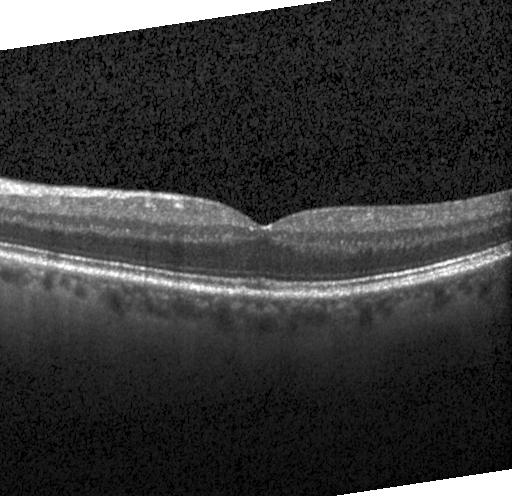 Instrument: Heidelberg Spectralis · through the macula · spectral-domain optical coherence tomography · retinal OCT cross-section — Impression: neither CNV, DME, nor drusen.